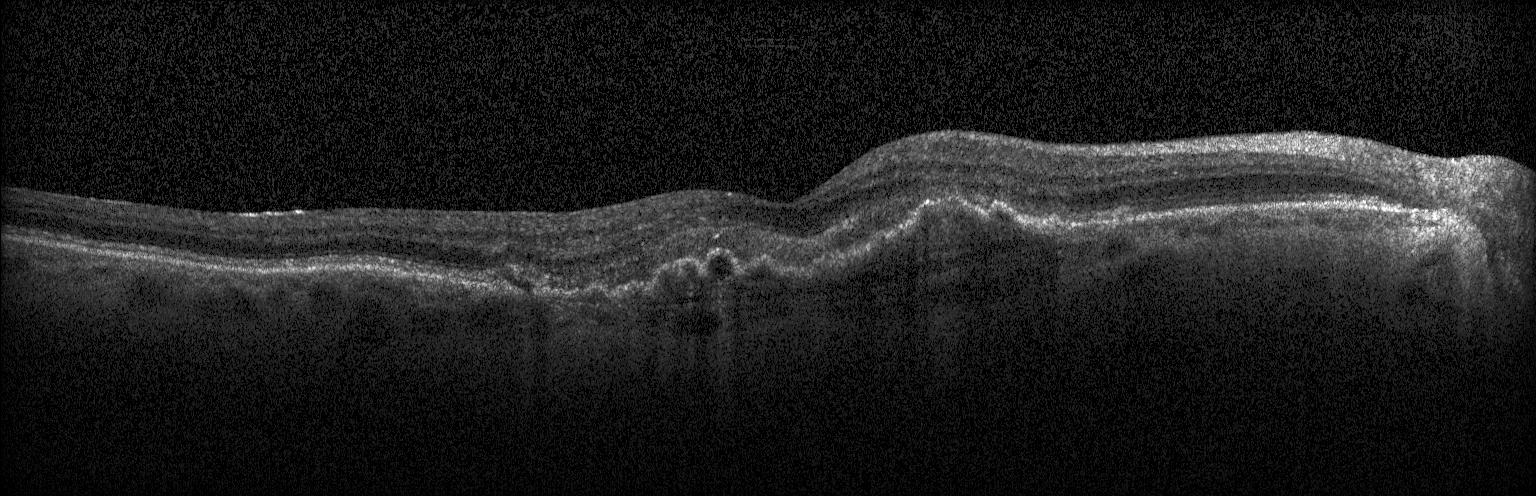 OCT B-scan — Diagnosis: choroidal neovascularization.